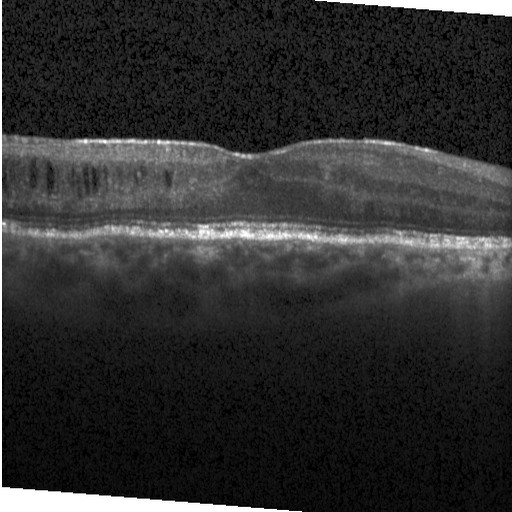

Retinal OCT cross-section showing diabetic macular edema (DME).